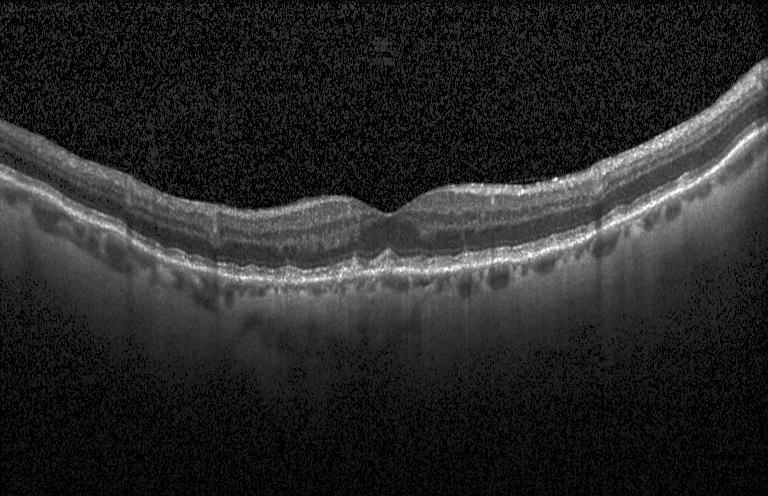
Assessment: sub-RPE drusenoid deposits.